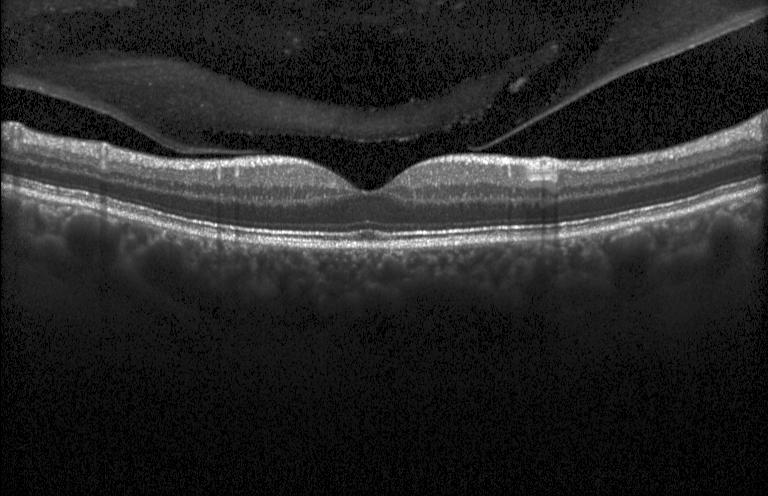 Impression: no choroidal neovascularization, diabetic macular edema, or drusen.